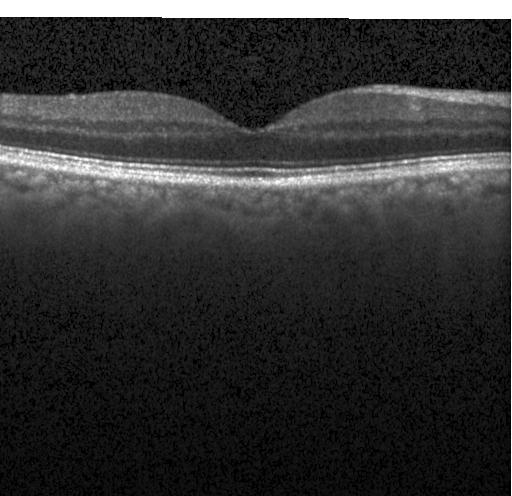
Neither choroidal neovascularization, diabetic macular edema, nor drusen.